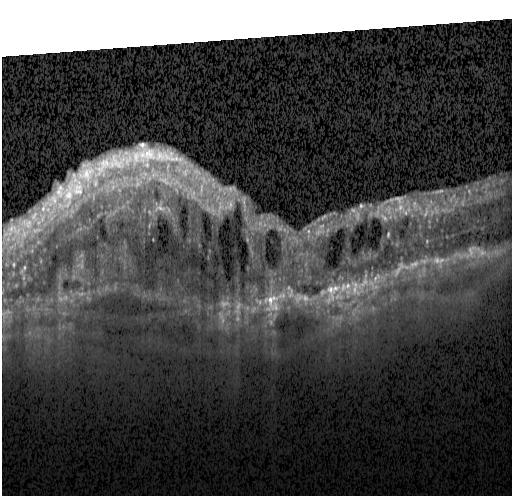 Instrument: Heidelberg Spectralis. Retinal OCT cross-section.
Impression: a choroidal neovascular membrane.